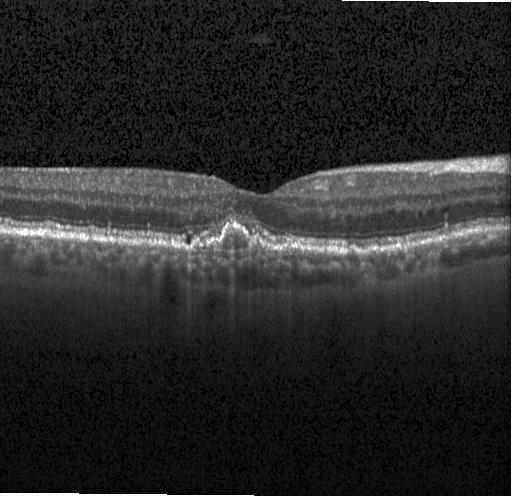 Optical coherence tomography scan — Diagnosis: choroidal neovascularization.